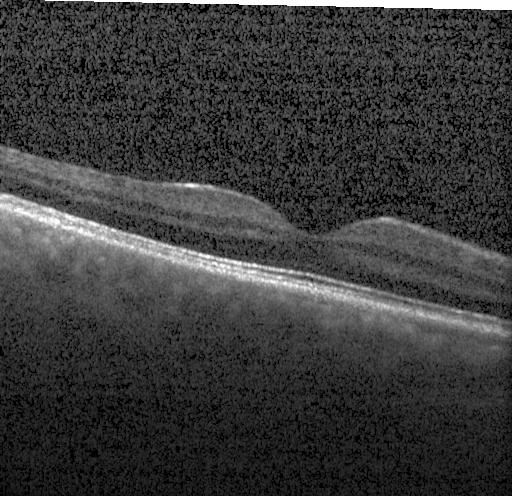 OCT line scan · centered on the fovea. Diagnosis: neither choroidal neovascularization, diabetic macular edema, nor drusen.